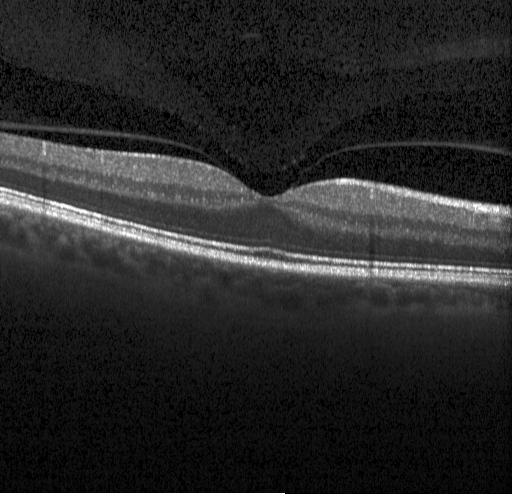 Optical coherence tomography B-scan
Macular OCT: neither CNV, DME, nor drusen.